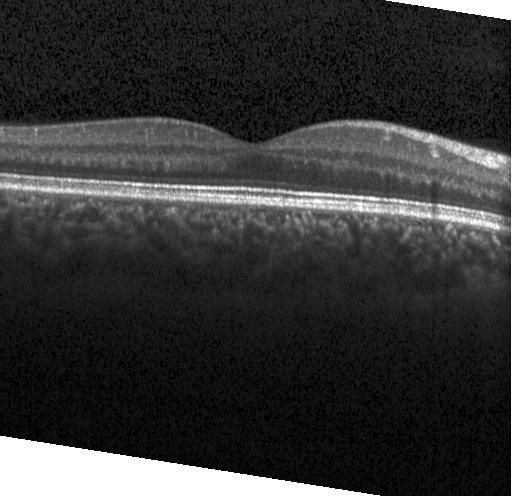
OCT line scan; acquired on a Heidelberg Spectralis — Finding: no evidence of choroidal neovascularization, diabetic macular edema, or drusen.